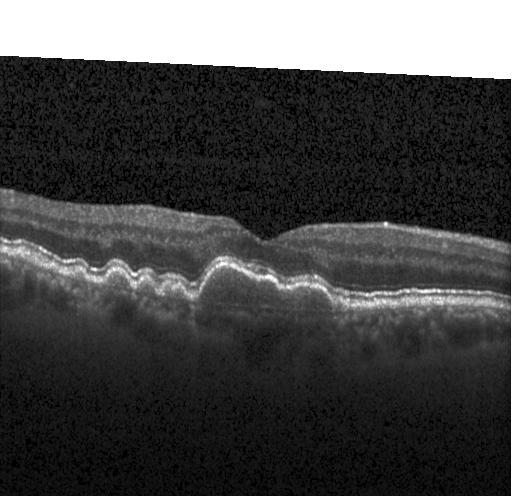
OCT B-scan. Heidelberg Spectralis. Spectral-domain OCT. Horizontal scan through the fovea. Assessment: sub-RPE drusenoid deposits.